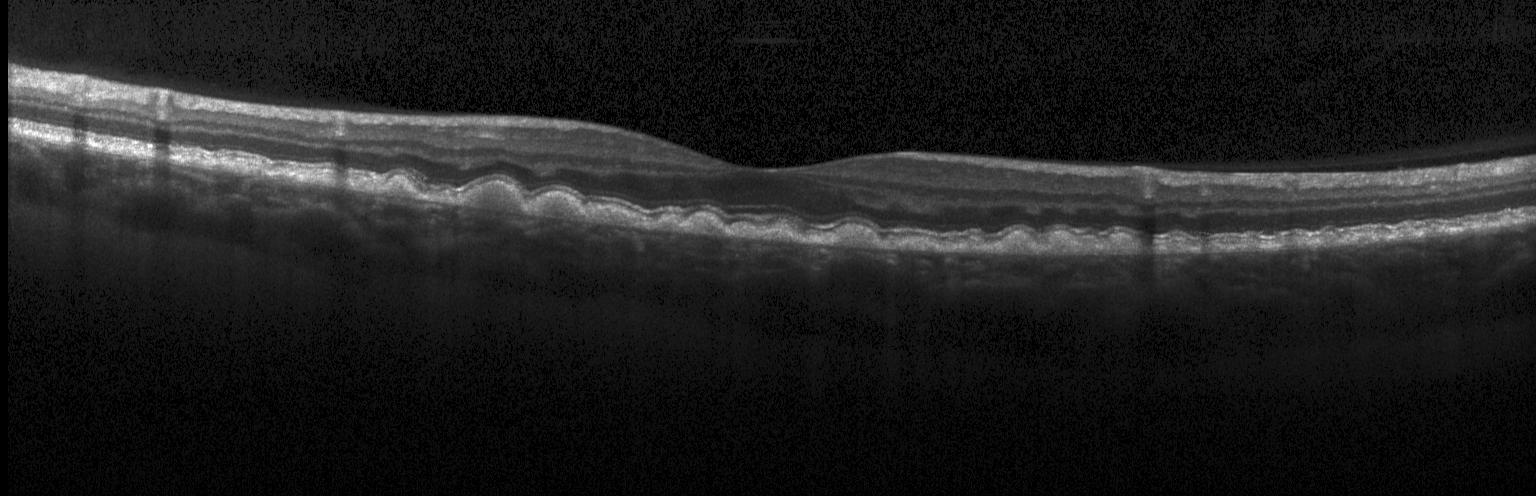 Optical coherence tomography scan; Heidelberg Spectralis; horizontal scan through the fovea.
The scan shows sub-RPE drusenoid deposits.